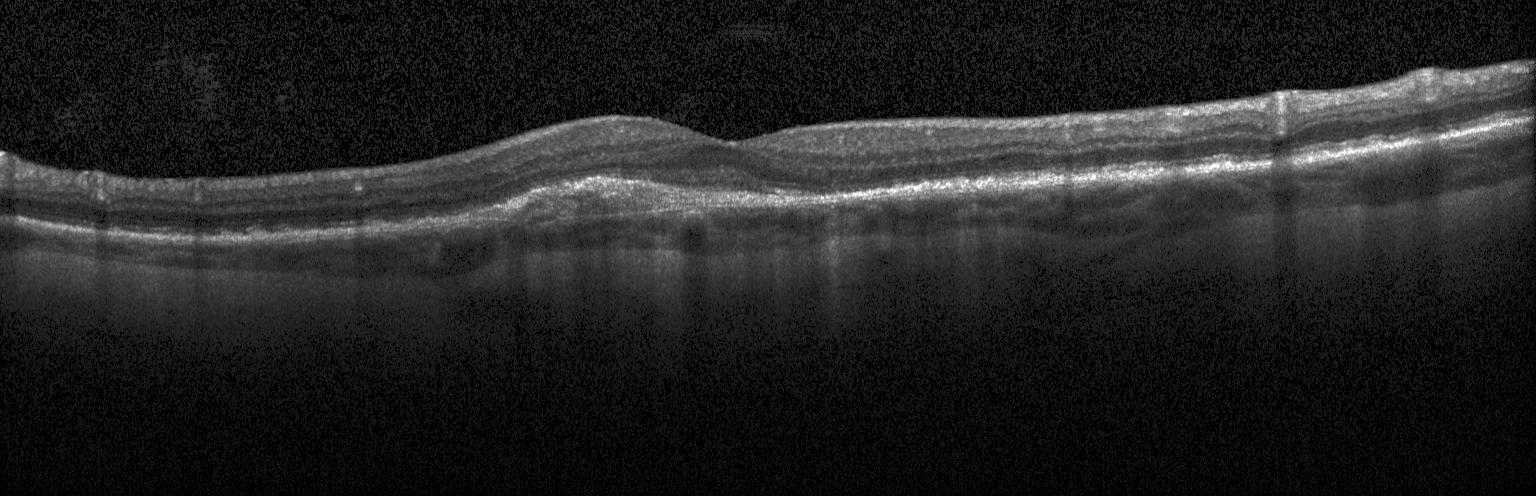 Optical coherence tomography B-scan — Assessment: choroidal neovascularization.